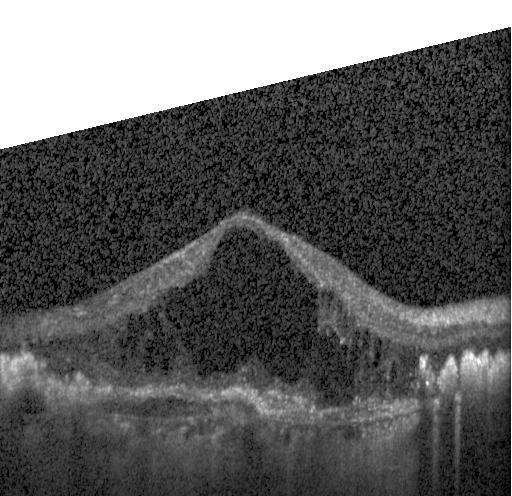

Heidelberg Spectralis, spectral-domain OCT, retinal OCT B-scan — Dx: choroidal neovascularization (CNV).